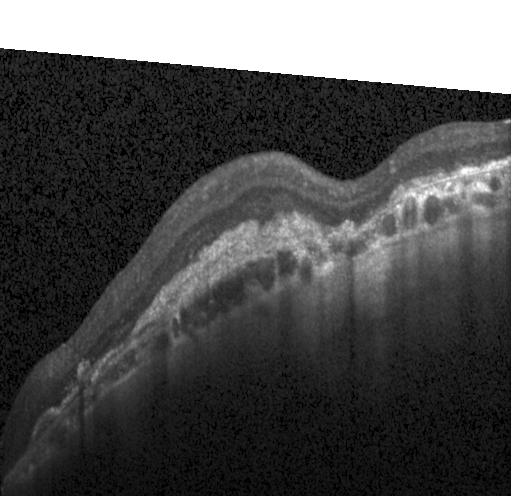 Through the macula; Heidelberg Spectralis; spectral-domain optical coherence tomography; optical coherence tomography scan
Finding: choroidal neovascularization (CNV).